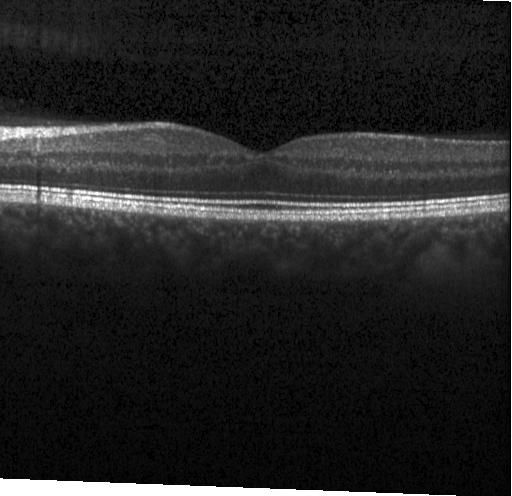 Diagnosis: no choroidal neovascularization, no diabetic macular edema, and no drusen.